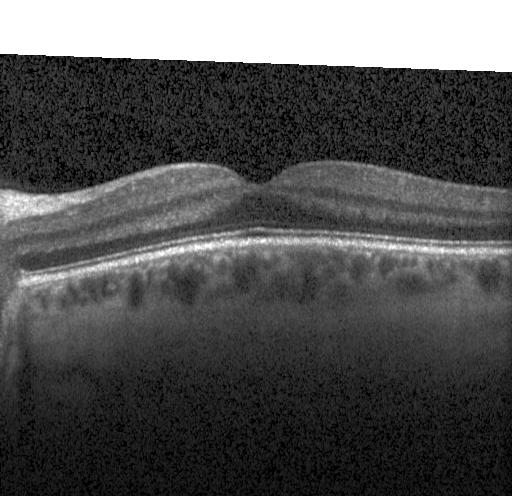

Heidelberg Spectralis OCT system, retinal OCT cross-section, SD-OCT
Impression: neither choroidal neovascularization, diabetic macular edema, nor drusen.